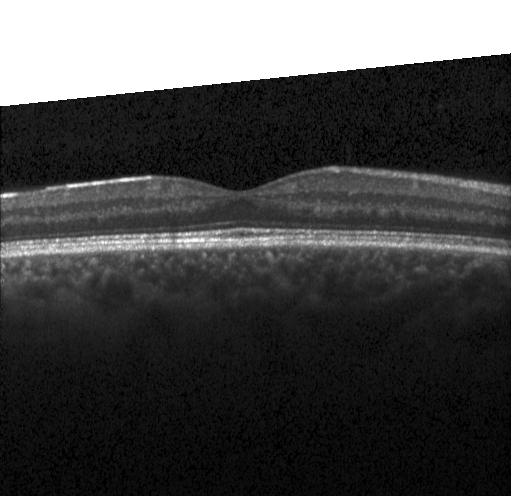

Spectral-domain OCT B-scan: no evidence of choroidal neovascularization, diabetic macular edema, or drusen.